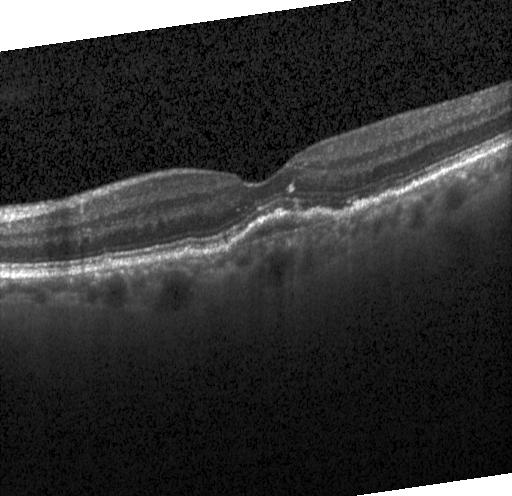 OCT B-scan. Dx: a choroidal neovascular membrane.